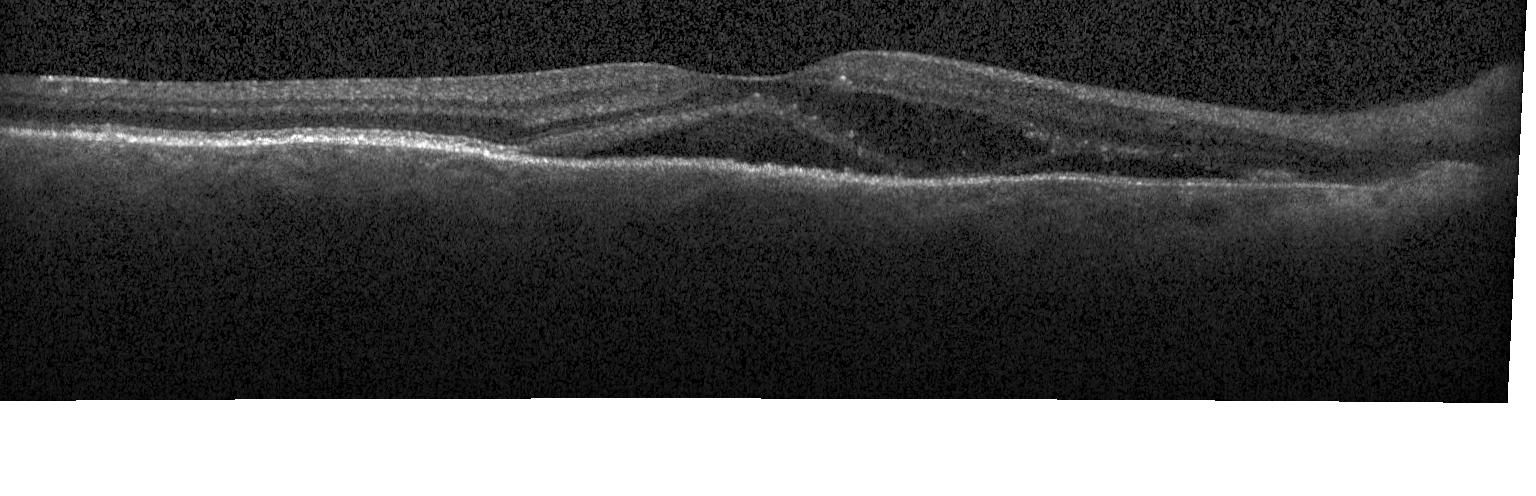

OCT line scan.
This B-scan demonstrates choroidal neovascularization.